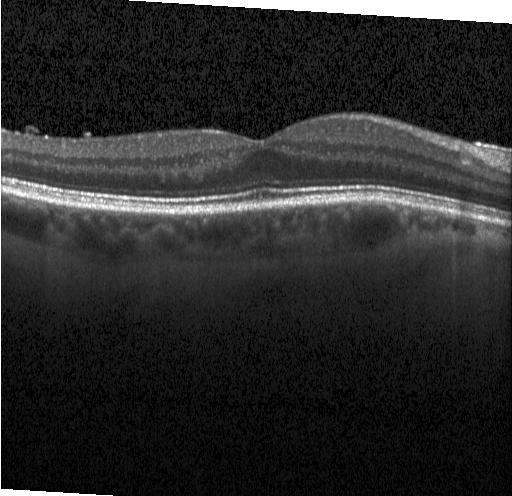

Assessment: no evidence of CNV, DME, or drusen.